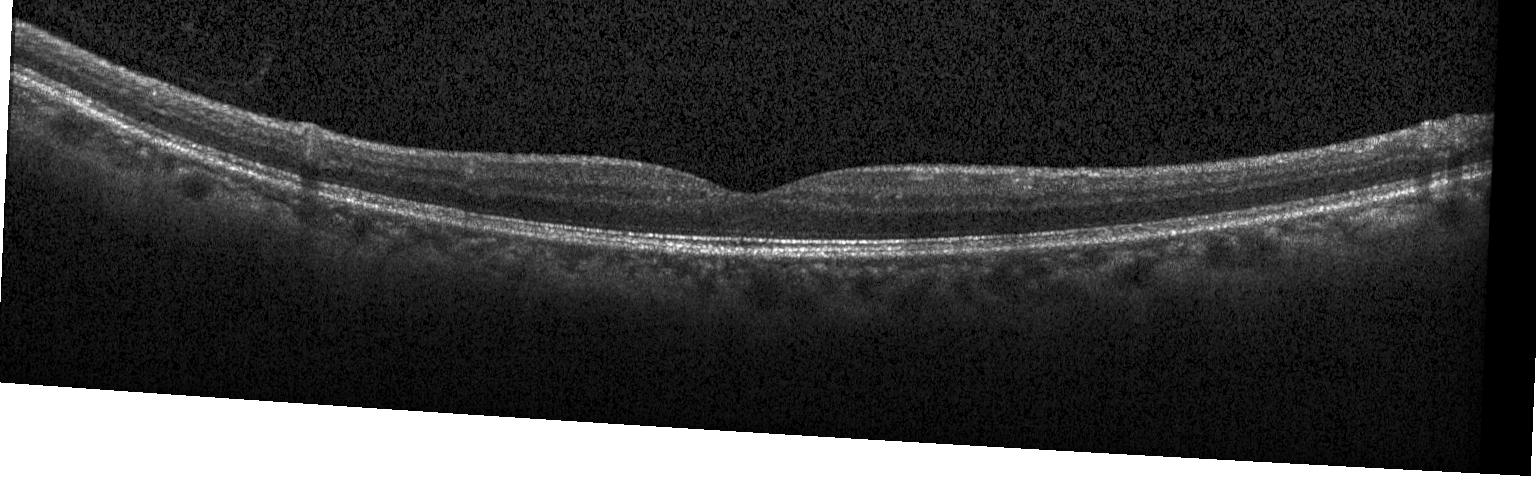 Centered on the fovea, spectral-domain OCT, instrument: Heidelberg Spectralis, OCT B-scan — Diagnosis: no choroidal neovascularization, no diabetic macular edema, and no drusen.